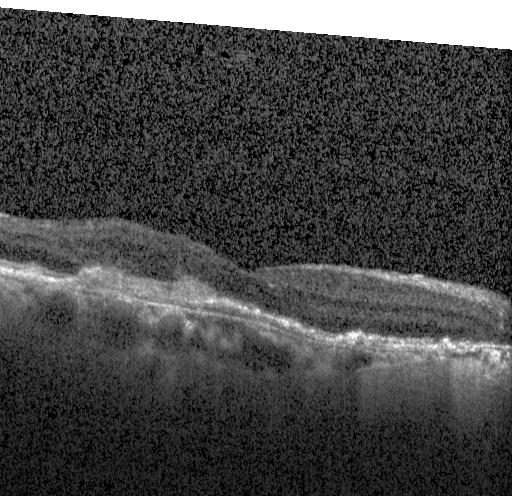

Retinal OCT B-scan. Diagnosis: a choroidal neovascular membrane.